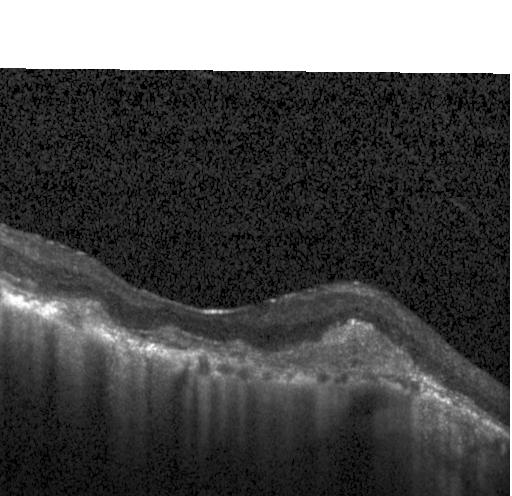 Optical coherence tomography scan, Heidelberg Spectralis OCT system, fovea-centered, spectral-domain OCT.
OCT finding: choroidal neovascularization (CNV).